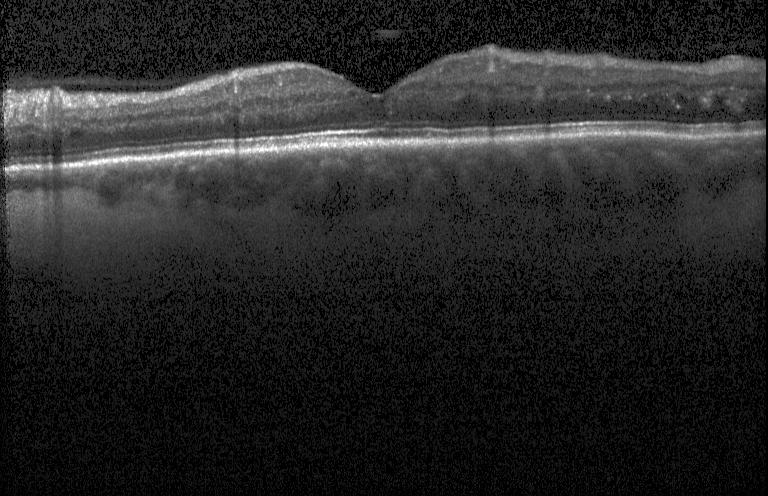
Macular OCT demonstrating diabetic macular edema.